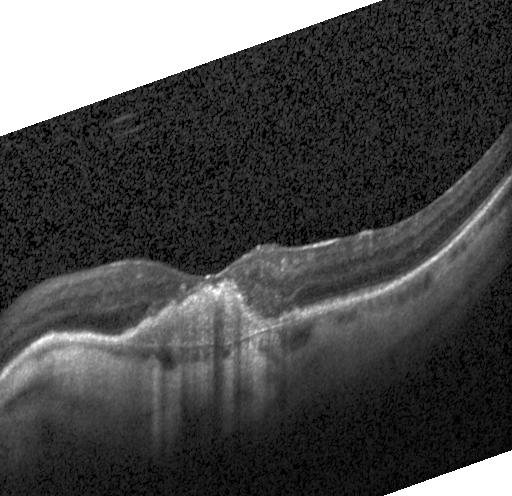 Impression: a choroidal neovascular membrane.